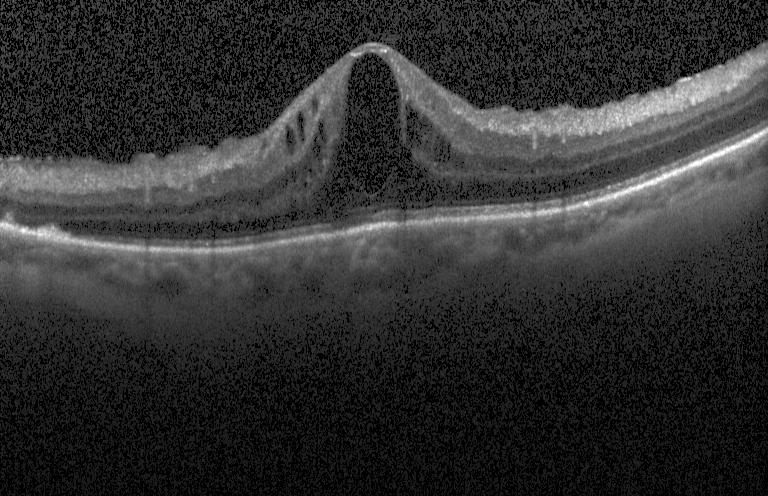

Finding: diabetic macular edema (DME).